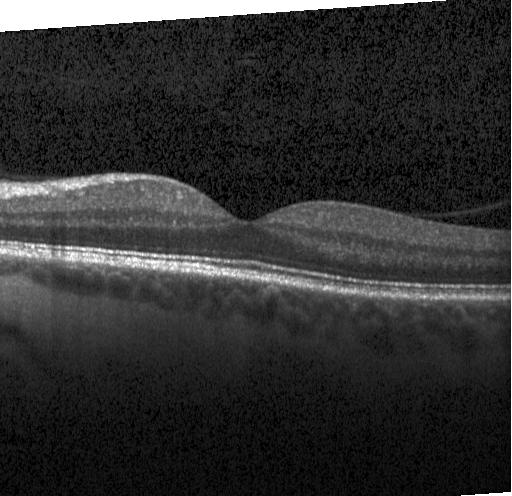 Macular OCT demonstrating no choroidal neovascularization, diabetic macular edema, or drusen.